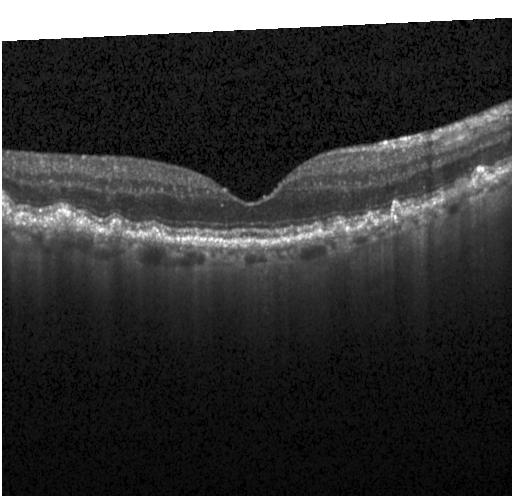 Fovea-centered, Heidelberg Spectralis, SD-OCT, optical coherence tomography B-scan.
Impression: sub-RPE drusenoid deposits.